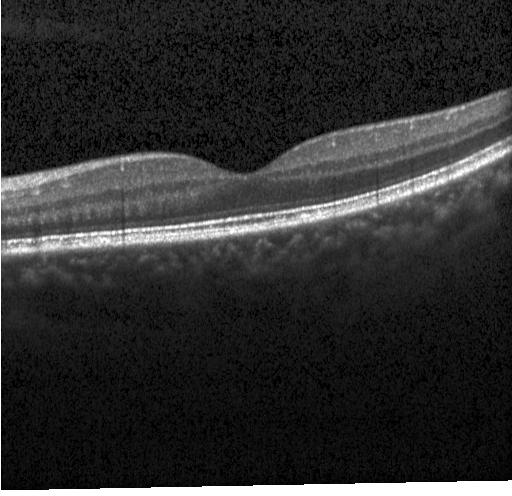 Macular OCT demonstrating no CNV, DME, or drusen.